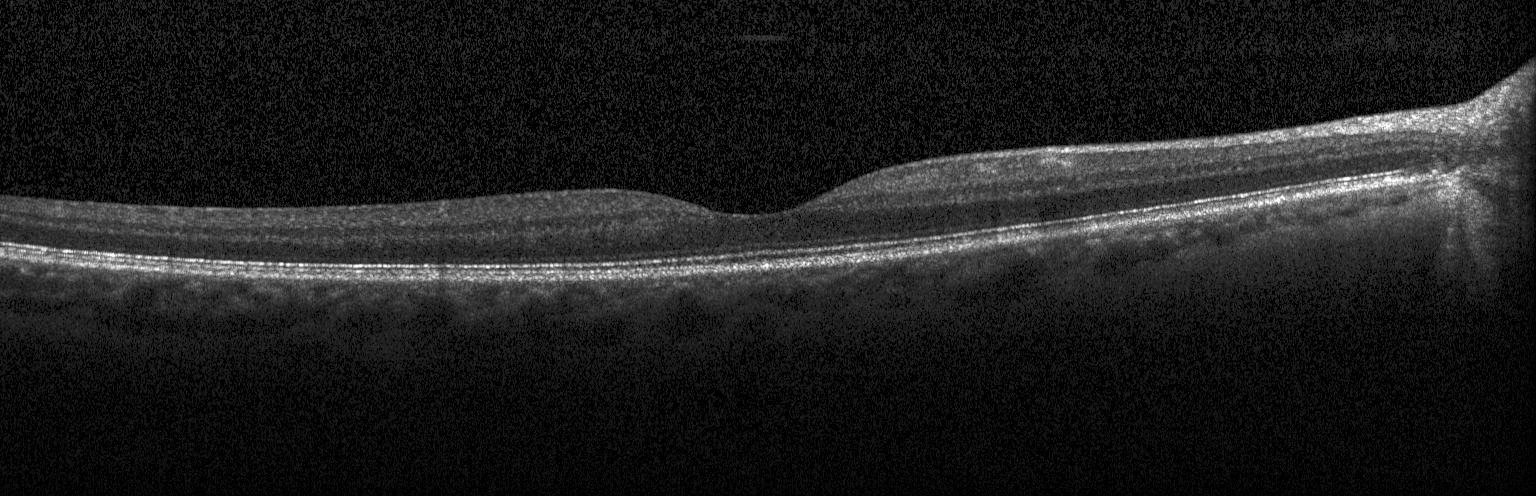
Diagnosis: neither choroidal neovascularization, diabetic macular edema, nor drusen.